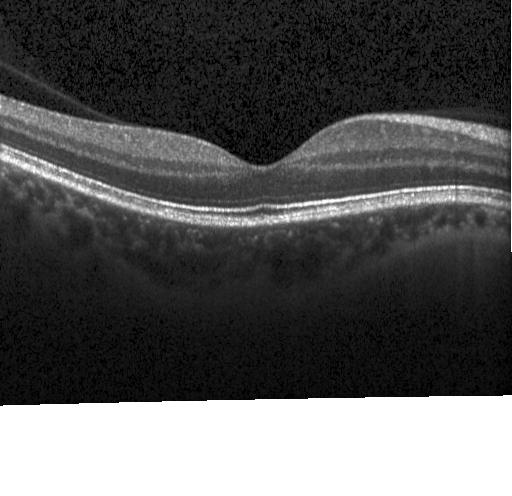 The scan shows neither choroidal neovascularization, diabetic macular edema, nor drusen.